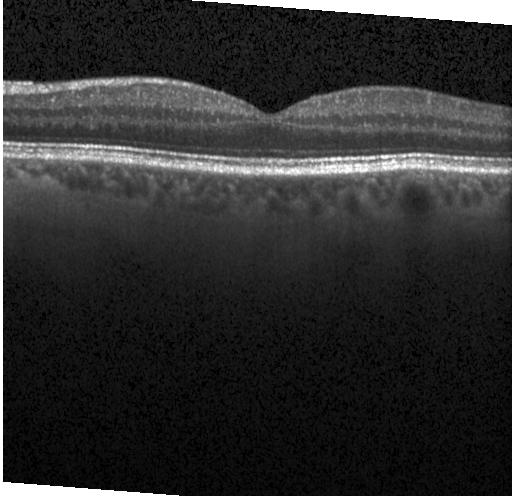 Dx: no choroidal neovascularization, no diabetic macular edema, and no drusen.